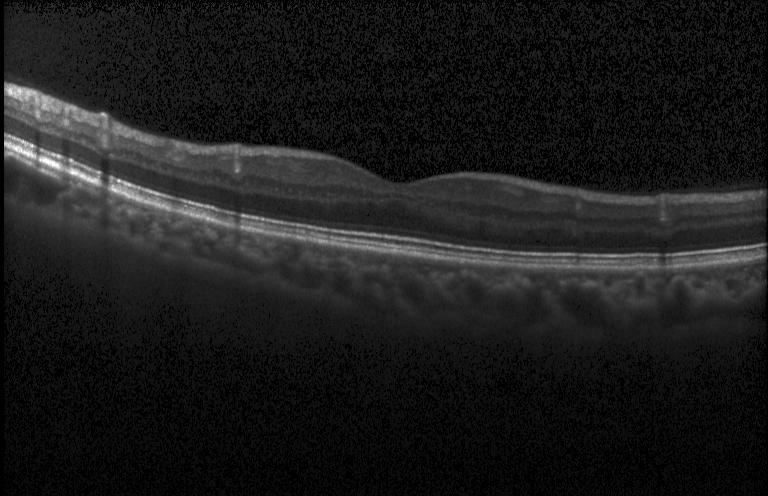 OCT line scan. OCT finding: no CNV, DME, or drusen.